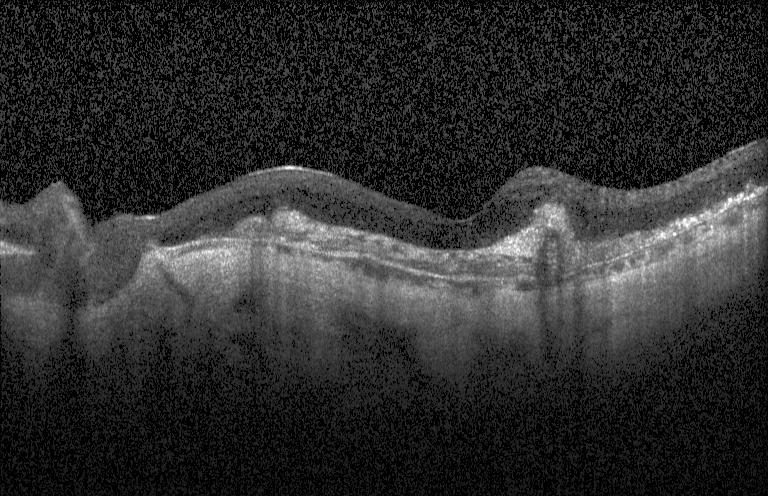 Macular OCT demonstrating a choroidal neovascular membrane.